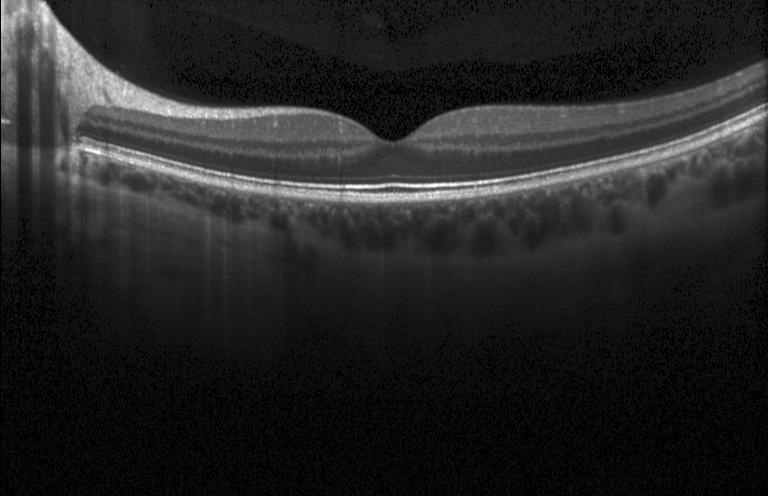
Macular OCT demonstrating neither choroidal neovascularization, diabetic macular edema, nor drusen.